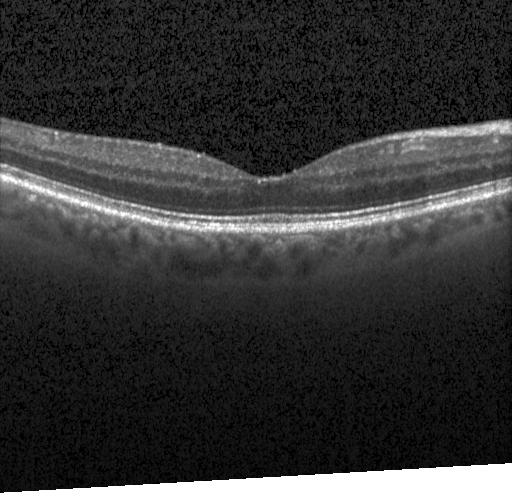 Macular OCT demonstrating no choroidal neovascularization, diabetic macular edema, or drusen.